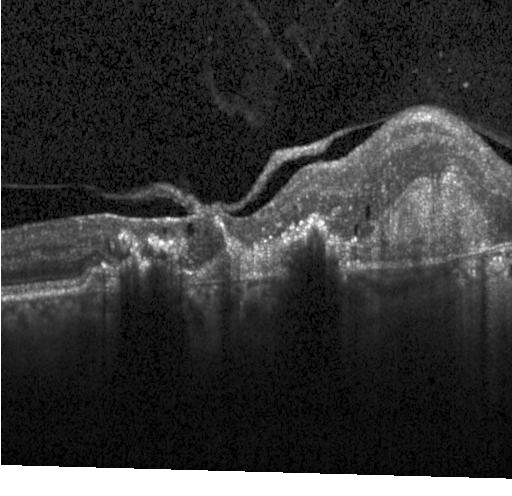

OCT line scan. The scan shows choroidal neovascularization (CNV).